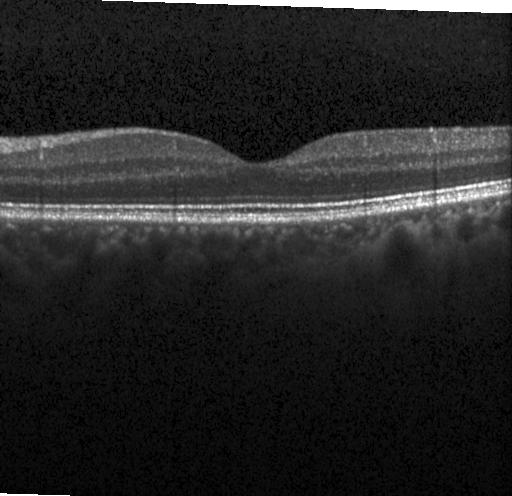 Retinal OCT B-scan, spectral-domain optical coherence tomography, centered on the fovea, Heidelberg Spectralis.
Neither CNV, DME, nor drusen.